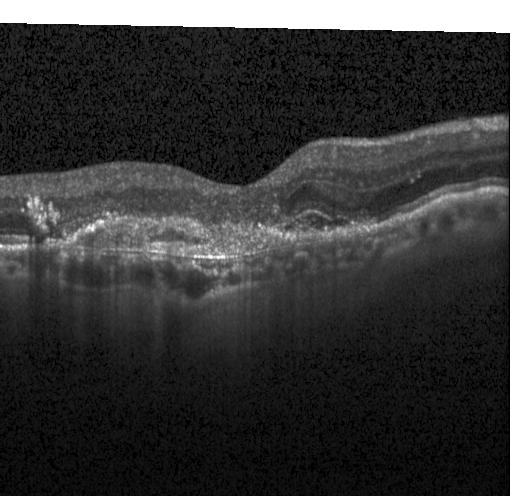

Retinal OCT cross-section, spectral-domain OCT.
Impression: a choroidal neovascular membrane.